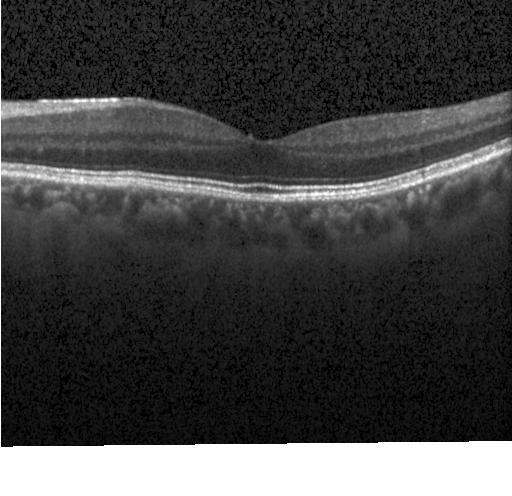 Optical coherence tomography B-scan
Diagnosis: neither choroidal neovascularization, diabetic macular edema, nor drusen.